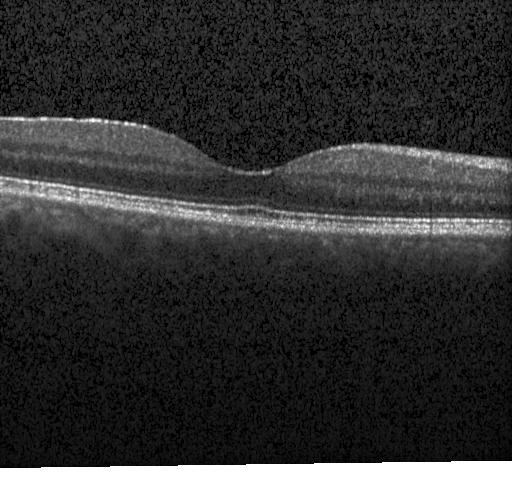

Impression: no evidence of CNV, DME, or drusen.